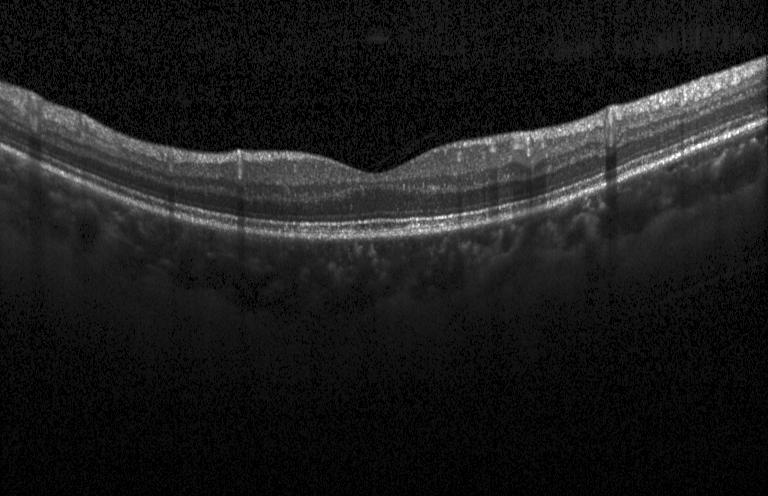 Finding: no evidence of CNV, DME, or drusen.